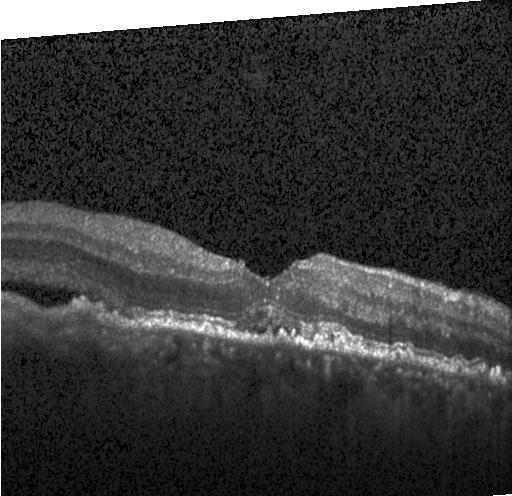

Spectral-domain OCT · acquired on a Heidelberg Spectralis · retinal OCT cross-section.
Assessment: choroidal neovascularization.